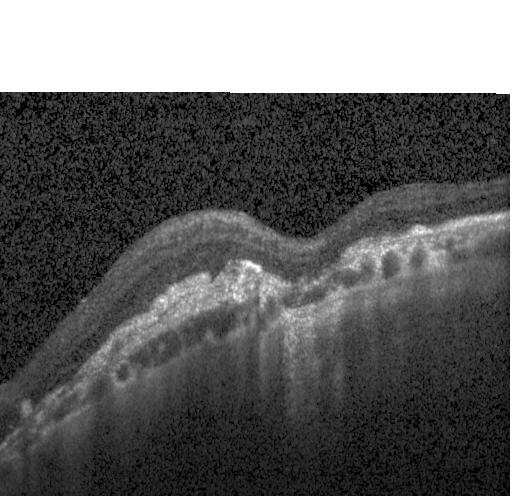 Fovea-centered. Heidelberg Spectralis. SD-OCT. Retinal OCT cross-section. Diagnosis: choroidal neovascularization.